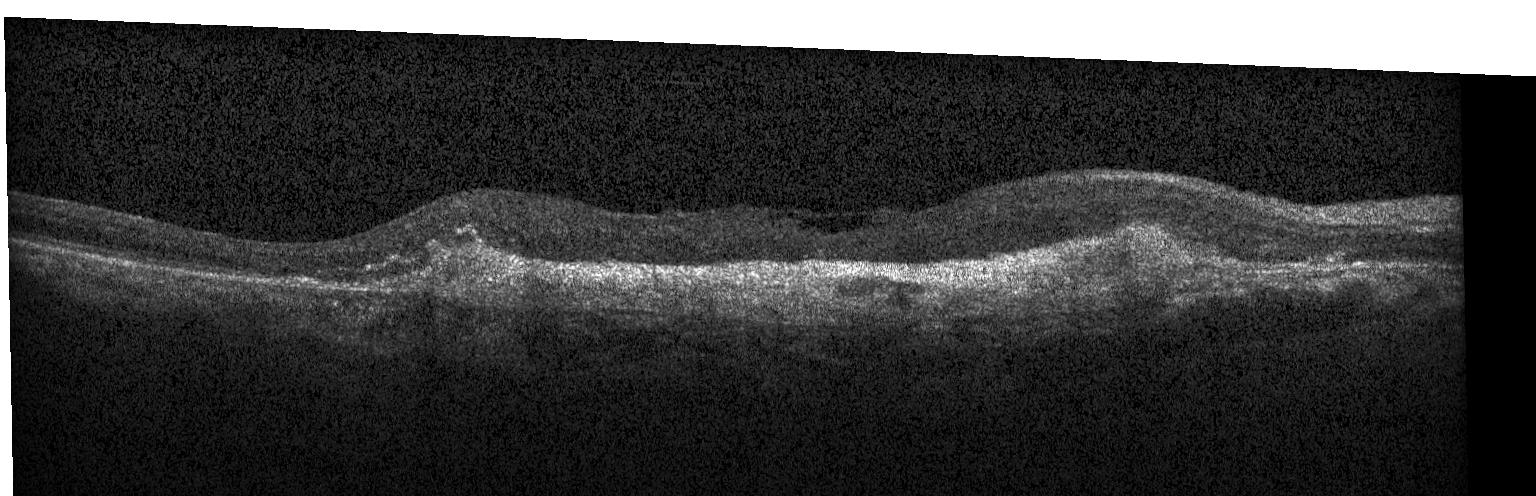

Heidelberg Spectralis · OCT line scan · fovea-centered · SD-OCT.
Diagnosis: a choroidal neovascular membrane.